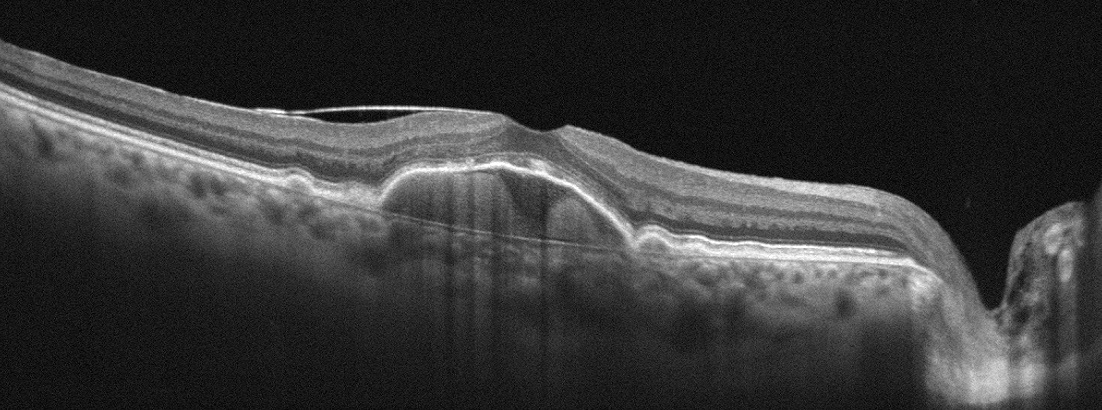

OCT line scan; instrument: Optovue Avanti RTVue XR
Dx: age-related macular degeneration (AMD).